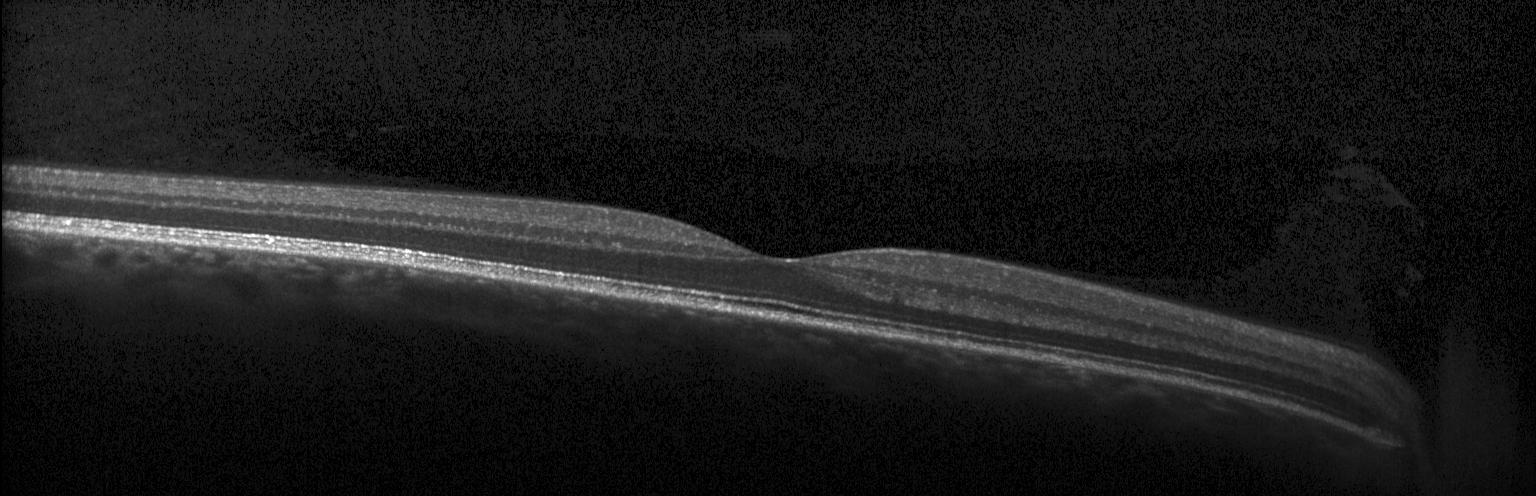
OCT B-scan · acquired on a Heidelberg Spectralis · macular scan · spectral-domain OCT. Neither CNV, DME, nor drusen.